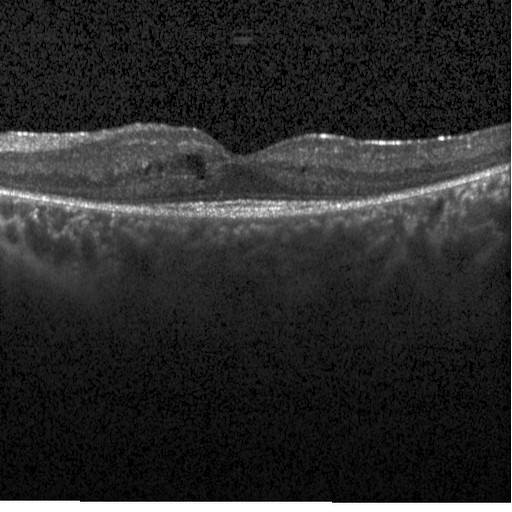 OCT line scan — Impression: diabetic macular edema.